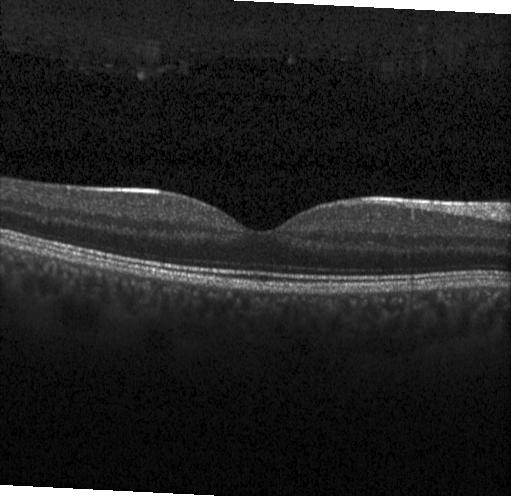

Optical coherence tomography B-scan. Dx: no choroidal neovascularization, no diabetic macular edema, and no drusen.